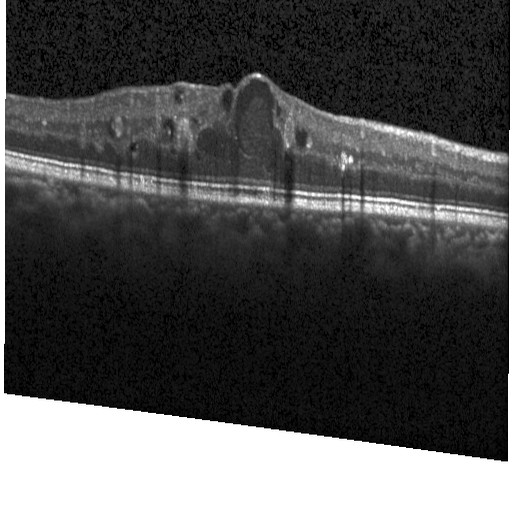

Diagnosis: diabetic macular edema.